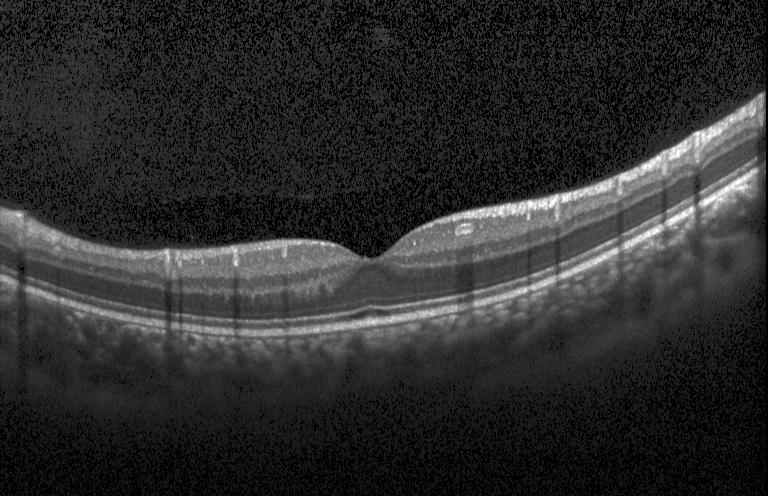

Retinal OCT B-scan. The scan shows no choroidal neovascularization, no diabetic macular edema, and no drusen.